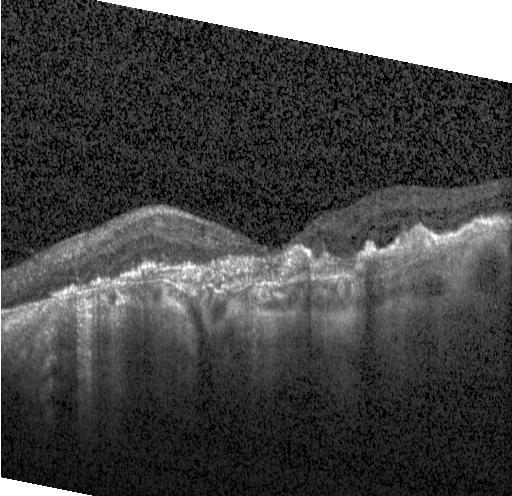
OCT line scan, horizontal scan through the fovea, Heidelberg Spectralis OCT system, spectral-domain optical coherence tomography.
Assessment: a choroidal neovascular membrane.